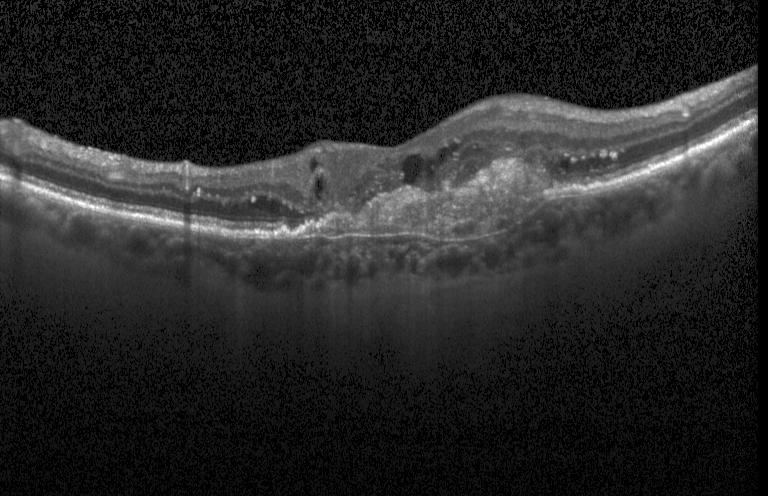

OCT line scan; acquired on a Heidelberg Spectralis — Impression: a choroidal neovascular membrane.